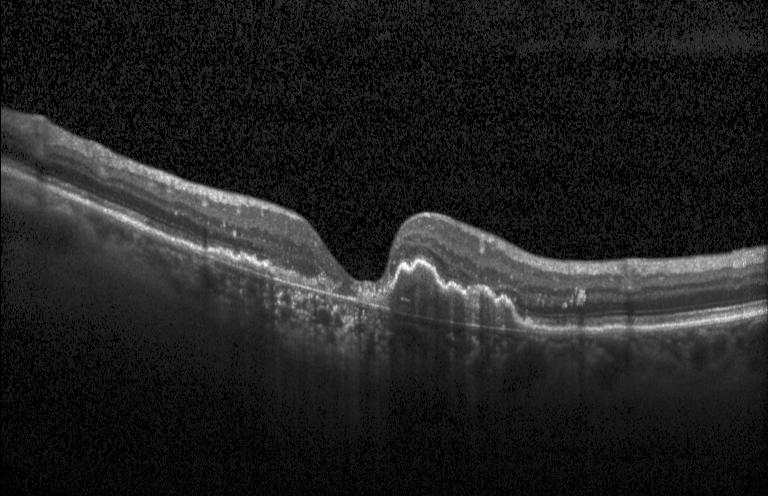 OCT scan showing a choroidal neovascular membrane.